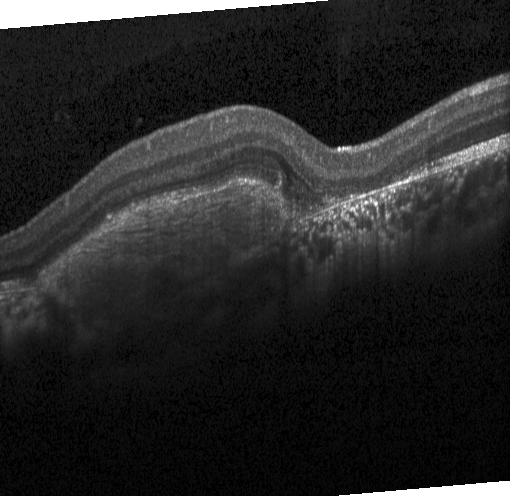

This B-scan demonstrates a choroidal neovascular membrane.